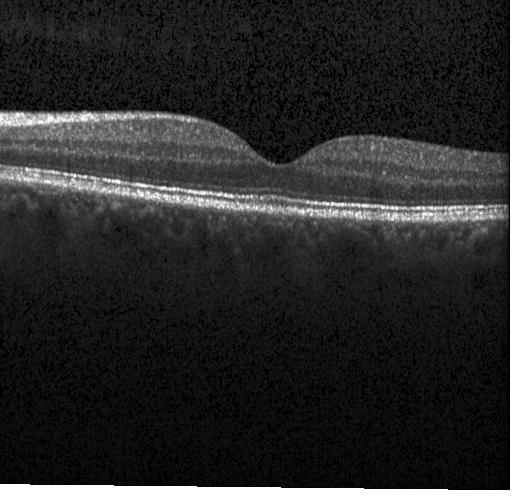

Macular OCT demonstrating no CNV, DME, or drusen.